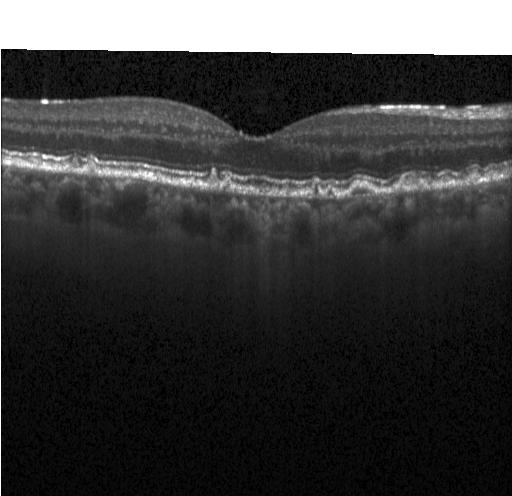
Macular OCT demonstrating sub-RPE drusenoid deposits.